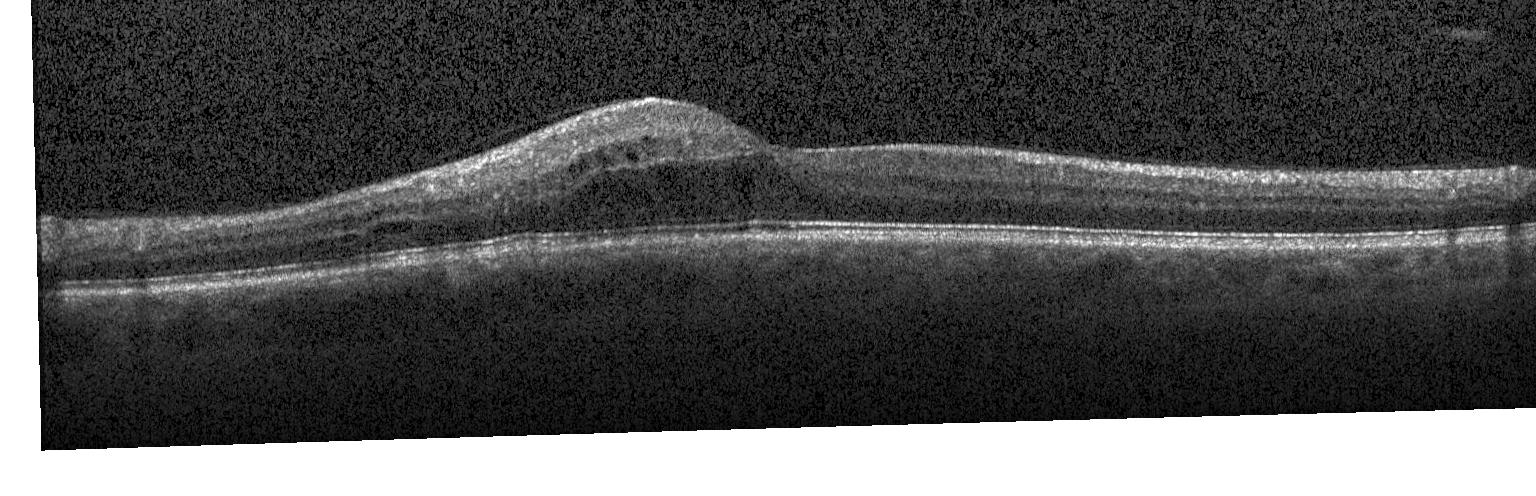
Optical coherence tomography B-scan; through the macula; acquired on a Heidelberg Spectralis; spectral-domain OCT. Impression: DME.